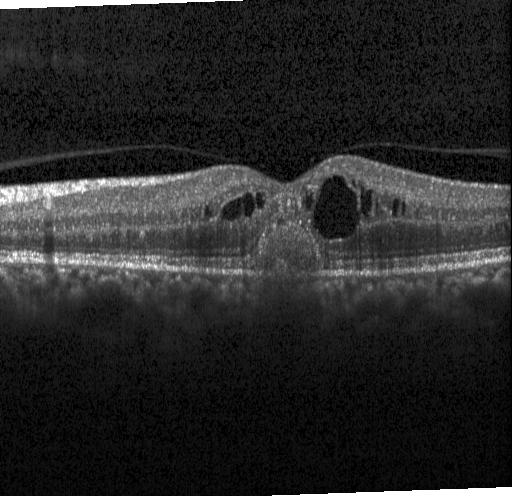
Optical coherence tomography B-scan. Impression: a choroidal neovascular membrane.